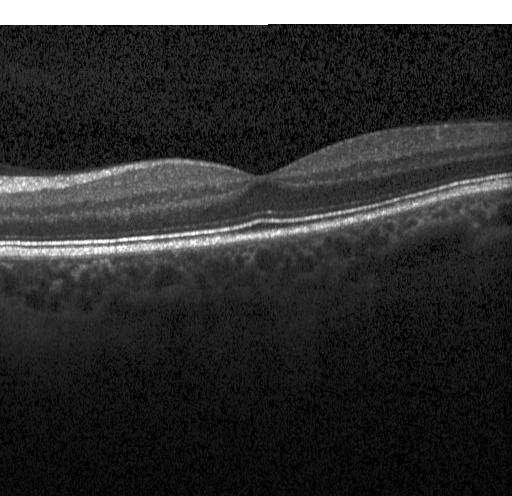

OCT line scan; instrument: Heidelberg Spectralis; horizontal scan through the fovea
Assessment: no choroidal neovascularization, diabetic macular edema, or drusen.